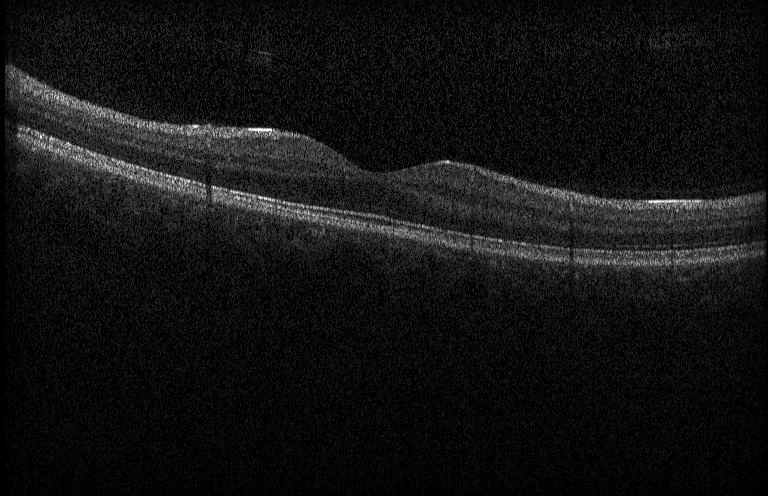

Assessment: neither CNV, DME, nor drusen.